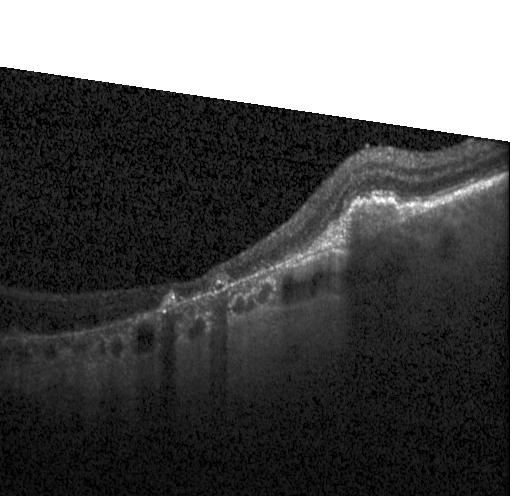
Optical coherence tomography scan. Spectral-domain optical coherence tomography. Heidelberg Spectralis. Centered on the fovea — OCT finding: a choroidal neovascular membrane.